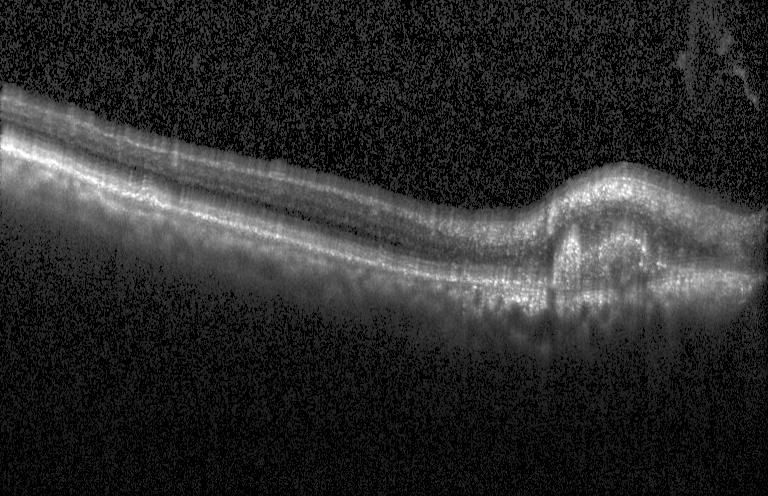
Finding: CNV.